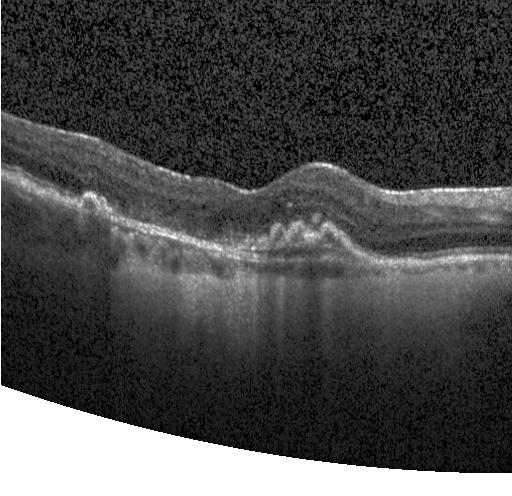

Acquired on a Heidelberg Spectralis, spectral-domain optical coherence tomography, OCT line scan
Impression: a choroidal neovascular membrane.